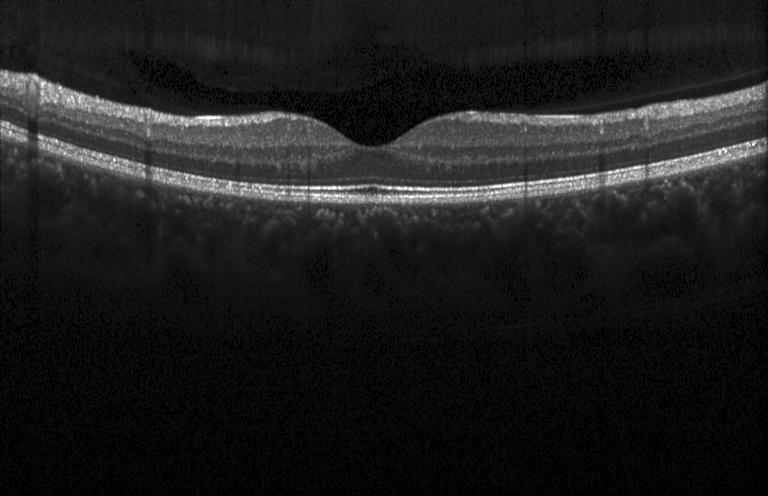

Horizontal scan through the fovea; retinal OCT cross-section; Heidelberg Spectralis OCT system
OCT finding: no evidence of CNV, DME, or drusen.